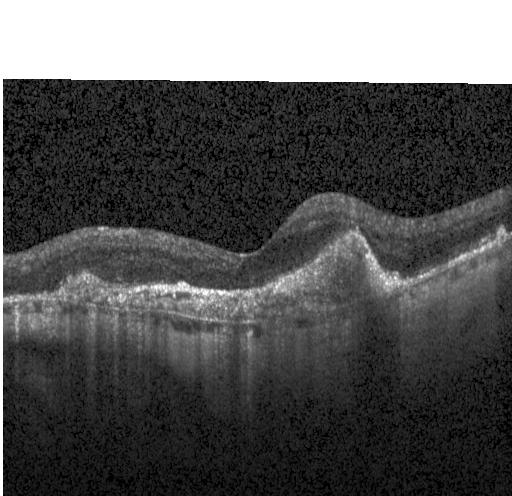

Instrument: Heidelberg Spectralis; optical coherence tomography B-scan
Impression: choroidal neovascularization.